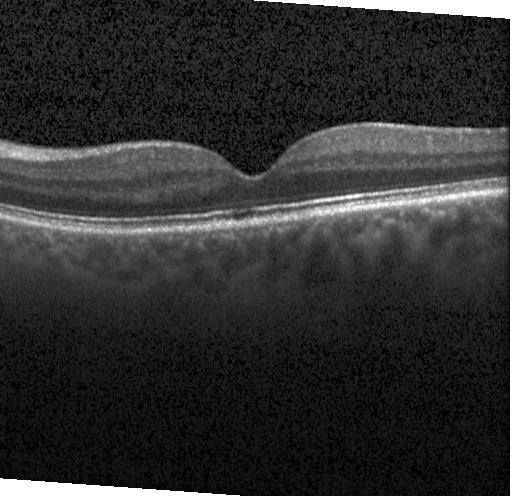
OCT finding: neither CNV, DME, nor drusen.